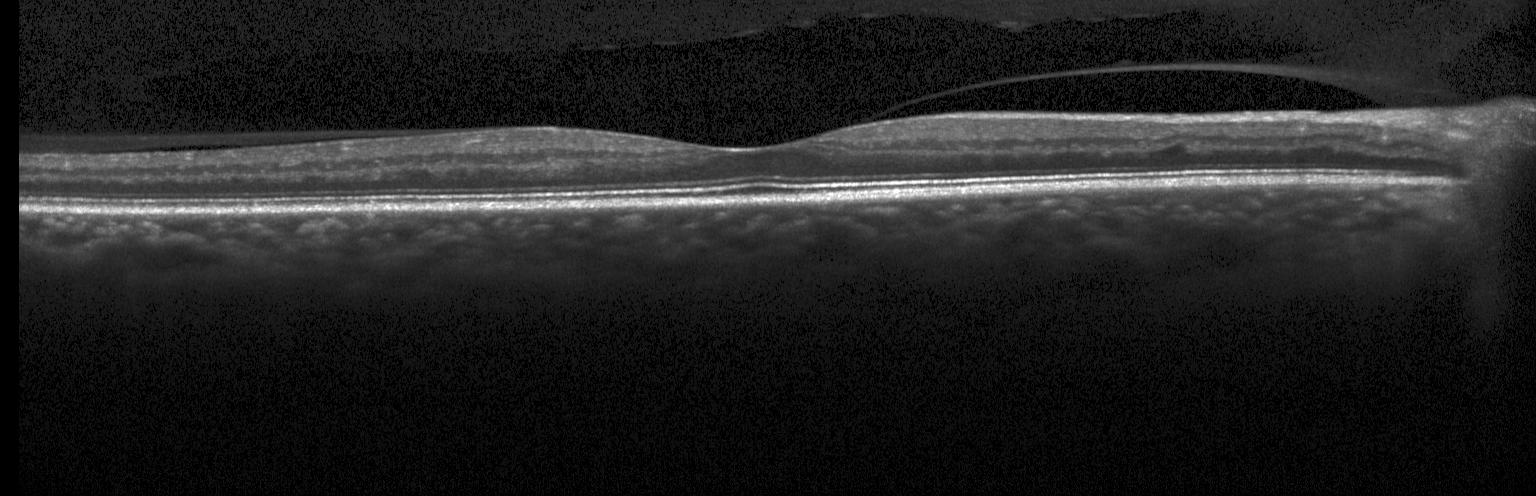

Through the macula. Heidelberg Spectralis. Optical coherence tomography scan.
Impression: neither choroidal neovascularization, diabetic macular edema, nor drusen.